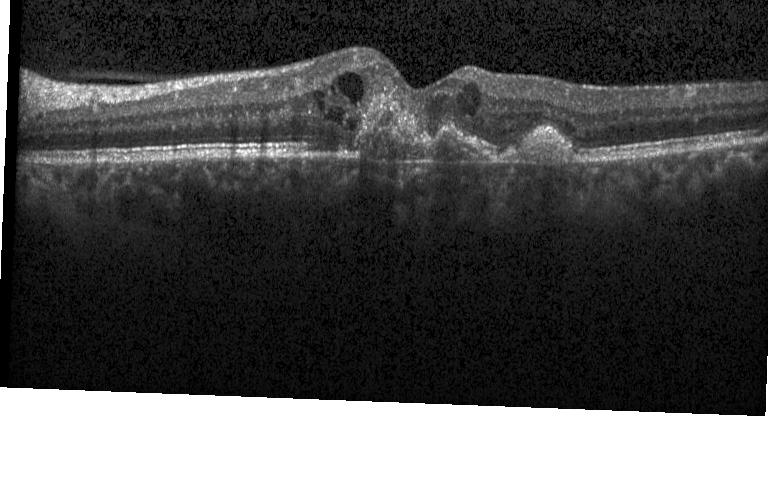 Optical coherence tomography B-scan; acquired on a Heidelberg Spectralis; SD-OCT.
Assessment: CNV.